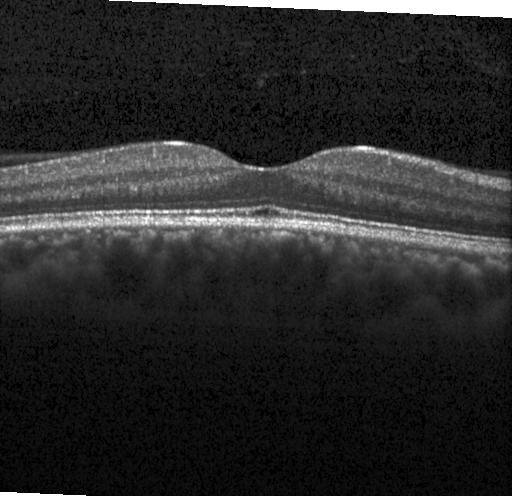 OCT B-scan — Finding: neither choroidal neovascularization, diabetic macular edema, nor drusen.